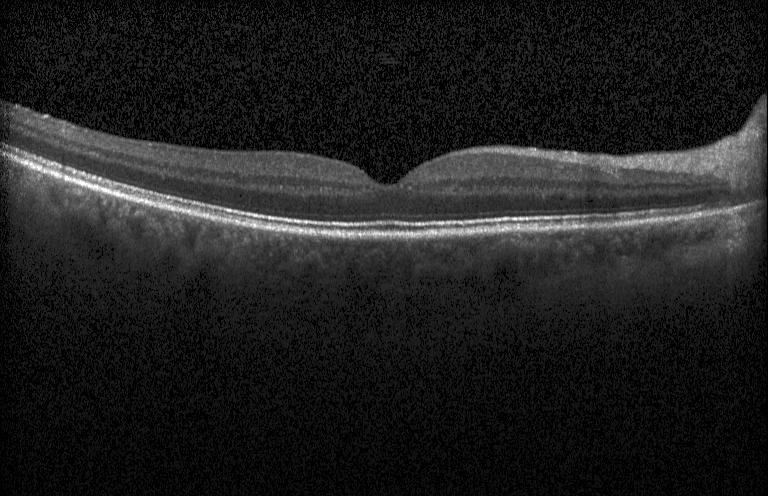

Instrument: Heidelberg Spectralis · optical coherence tomography B-scan · centered on the fovea · SD-OCT
The scan shows no choroidal neovascularization, no diabetic macular edema, and no drusen.